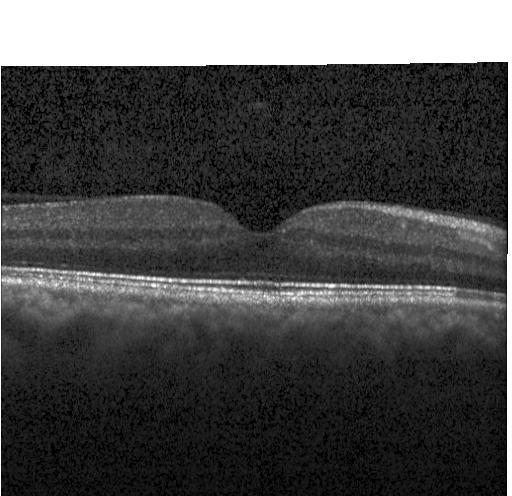 This B-scan demonstrates no CNV, no DME, and no drusen.